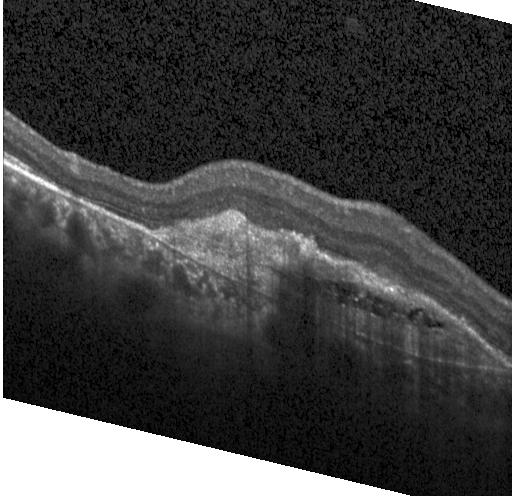
The scan shows choroidal neovascularization (CNV).